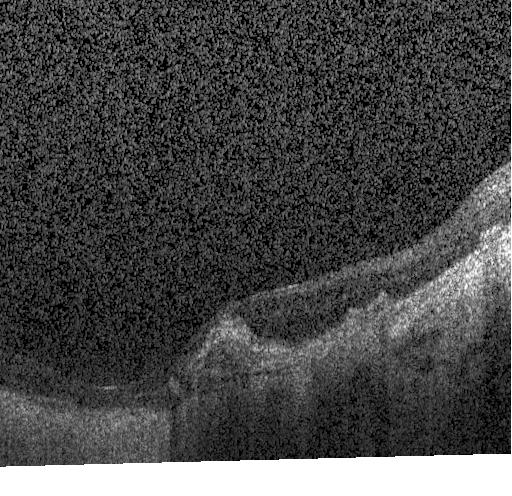

Finding: CNV.